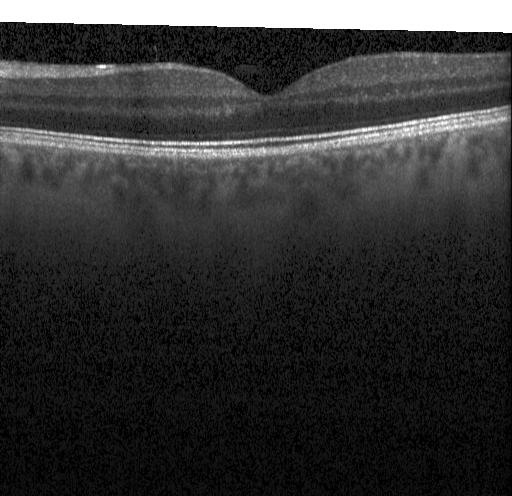

OCT B-scan; Heidelberg Spectralis — Neither CNV, DME, nor drusen.